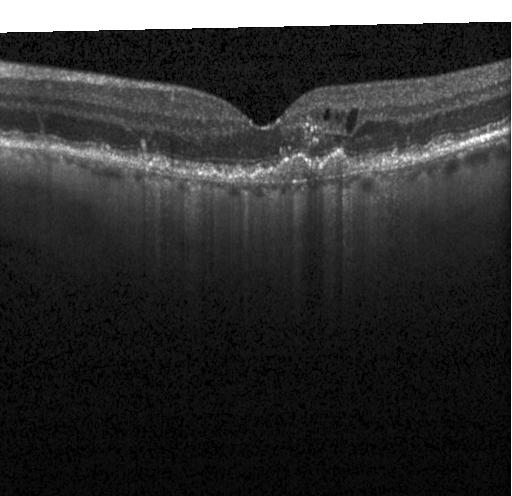
Retinal OCT cross-section. SD-OCT. Macular scan — Finding: CNV.